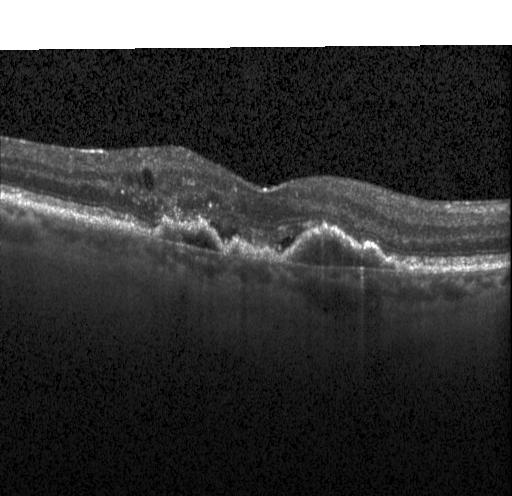

Optical coherence tomography scan, spectral-domain OCT. Finding: CNV.